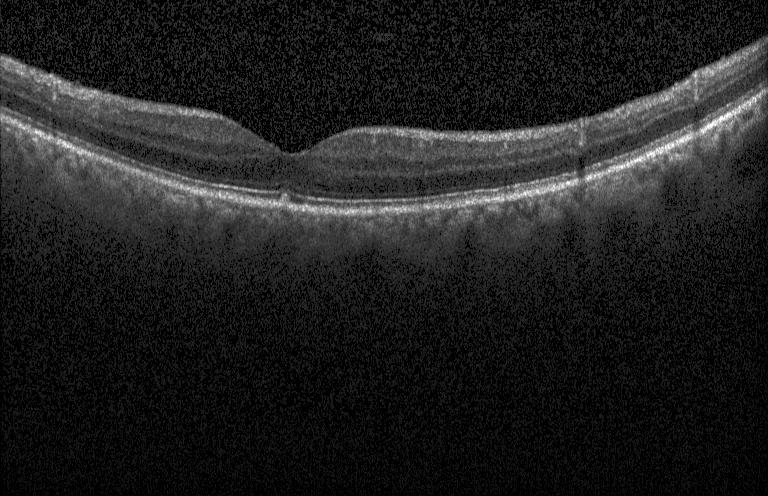
SD-OCT. OCT B-scan
Assessment: sub-RPE drusenoid deposits.